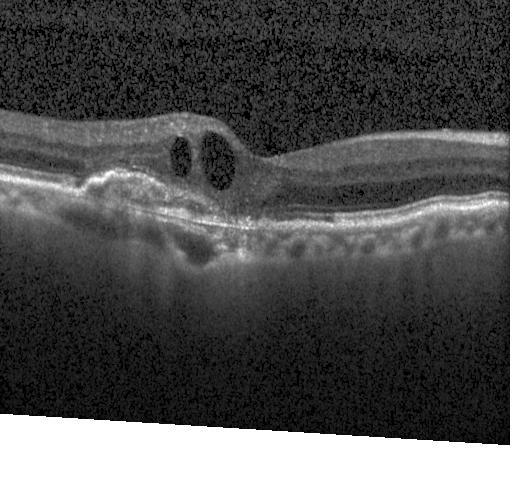
Macular OCT demonstrating CNV.